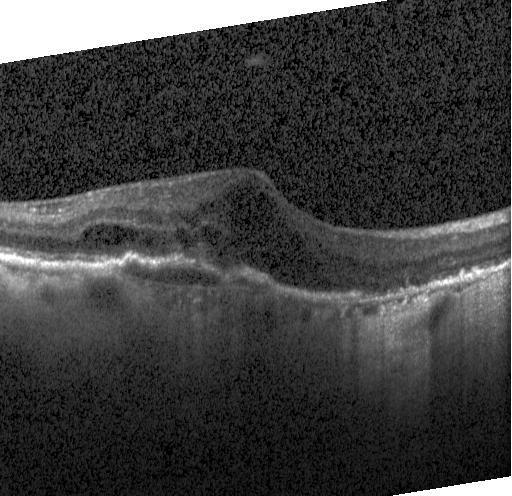 Macular OCT: a choroidal neovascular membrane.